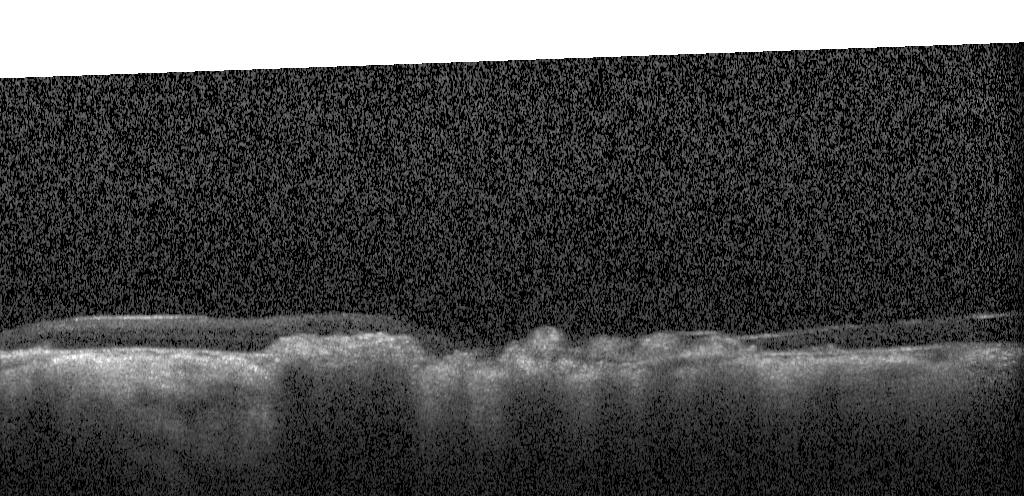
Macular scan, OCT B-scan.
The scan shows a choroidal neovascular membrane.